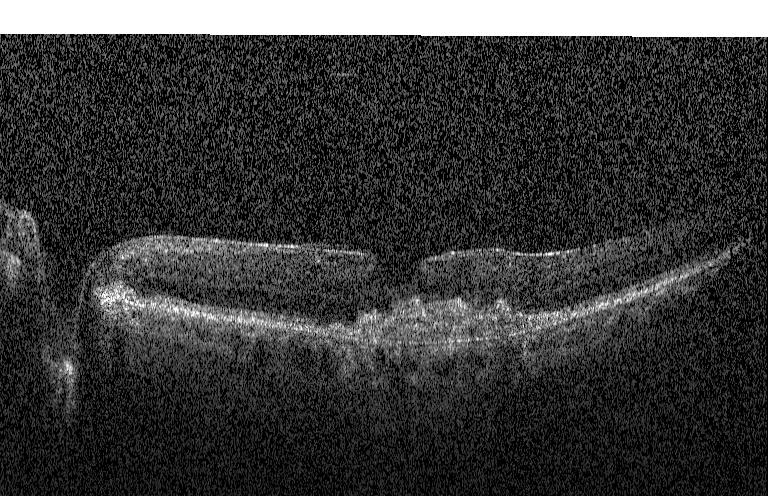 OCT line scan. A choroidal neovascular membrane.